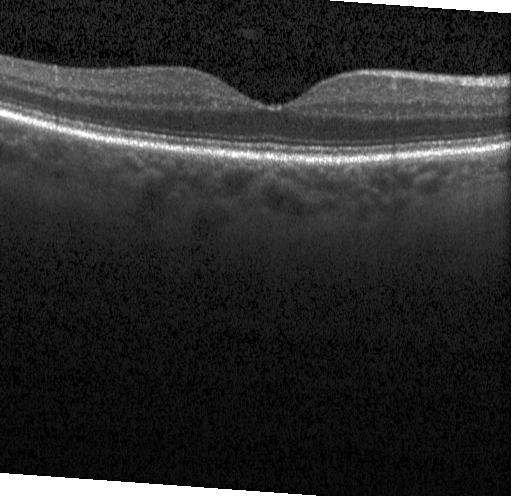
Retinal OCT cross-section. Assessment: no choroidal neovascularization, no diabetic macular edema, and no drusen.